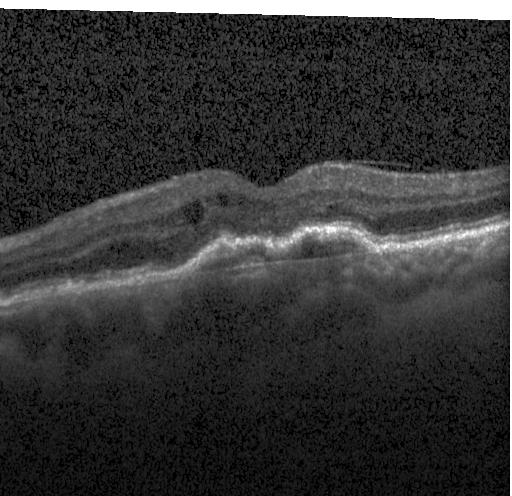 Acquired on a Heidelberg Spectralis. Retinal OCT B-scan. Spectral-domain optical coherence tomography.
Dx: a choroidal neovascular membrane.